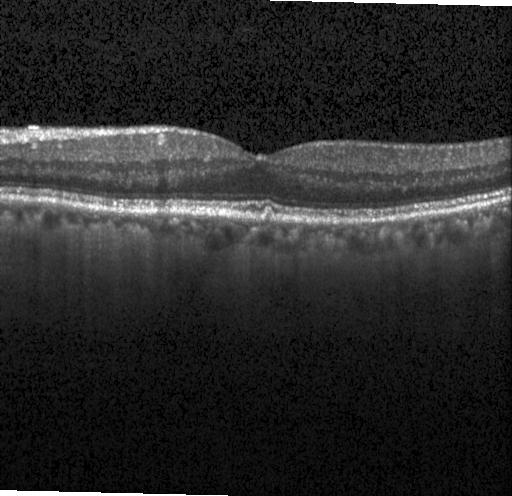
Diagnosis: sub-RPE drusenoid deposits.